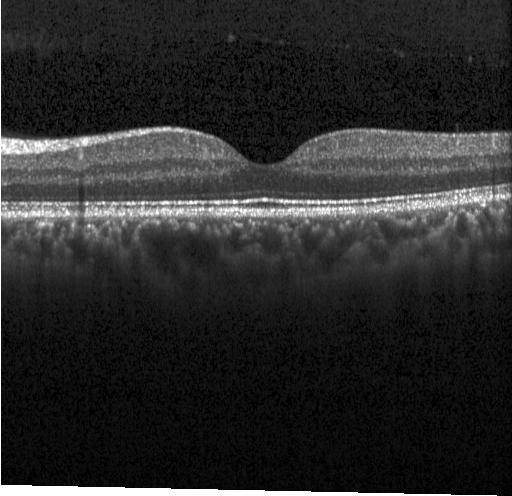 Optical coherence tomography scan. Heidelberg Spectralis OCT system. Assessment: neither CNV, DME, nor drusen.